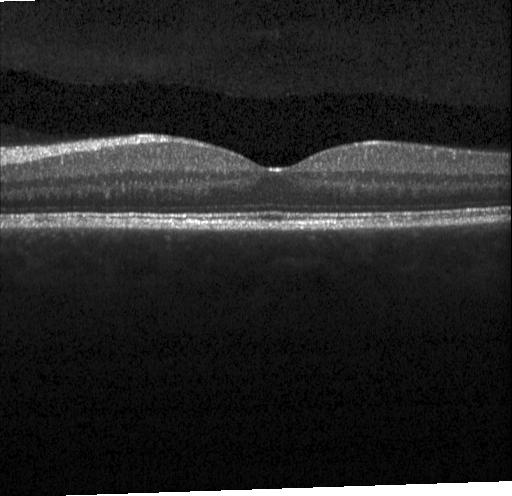
Spectral-domain OCT. Retinal OCT cross-section. Instrument: Heidelberg Spectralis. Horizontal scan through the fovea. Diagnosis: no choroidal neovascularization, diabetic macular edema, or drusen.